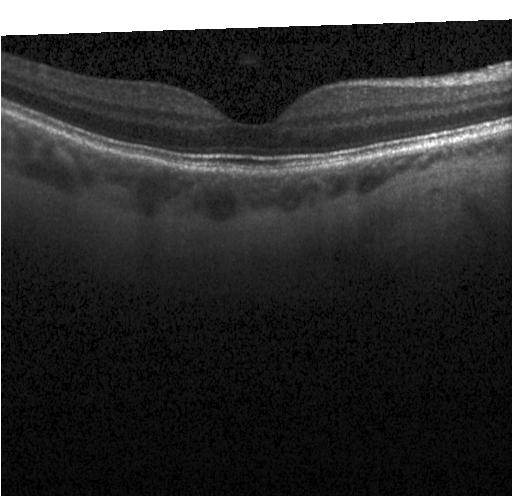

Horizontal scan through the fovea · optical coherence tomography scan — Impression: no evidence of CNV, DME, or drusen.